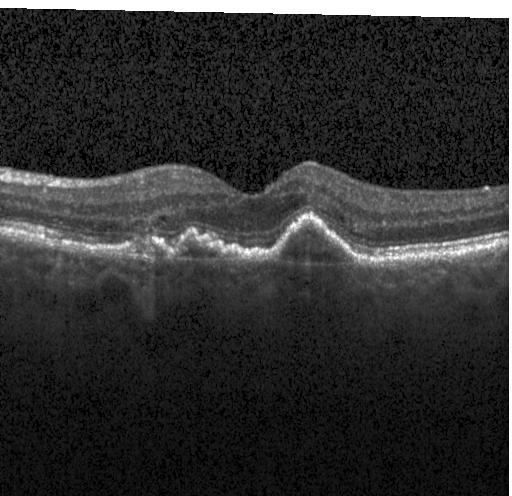
This B-scan demonstrates choroidal neovascularization (CNV).